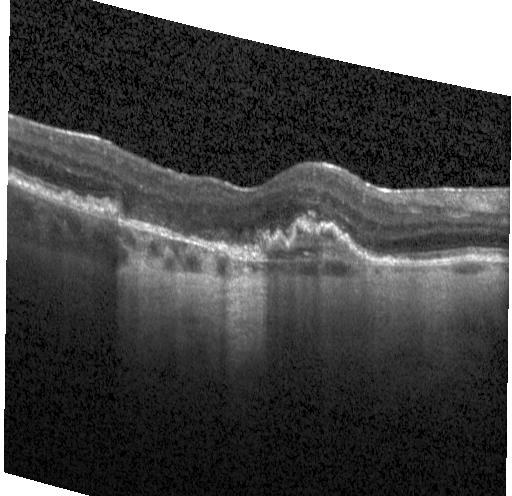
Retinal OCT cross-section; Heidelberg Spectralis OCT system; centered on the fovea; spectral-domain optical coherence tomography.
CNV.